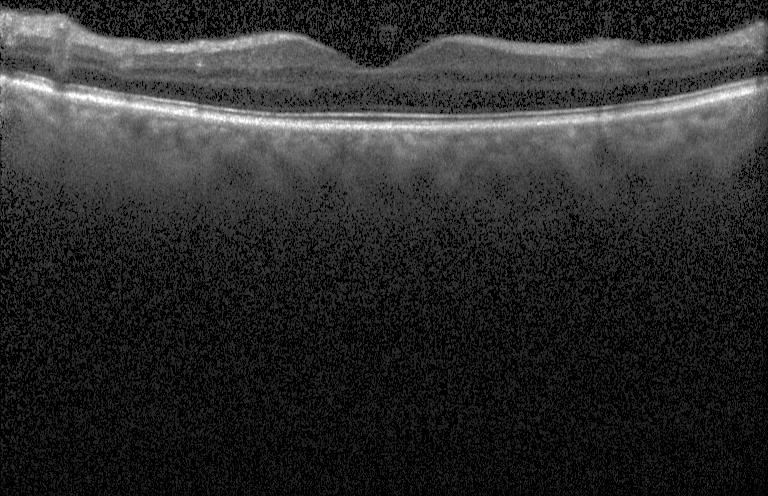 This B-scan demonstrates no evidence of CNV, DME, or drusen.